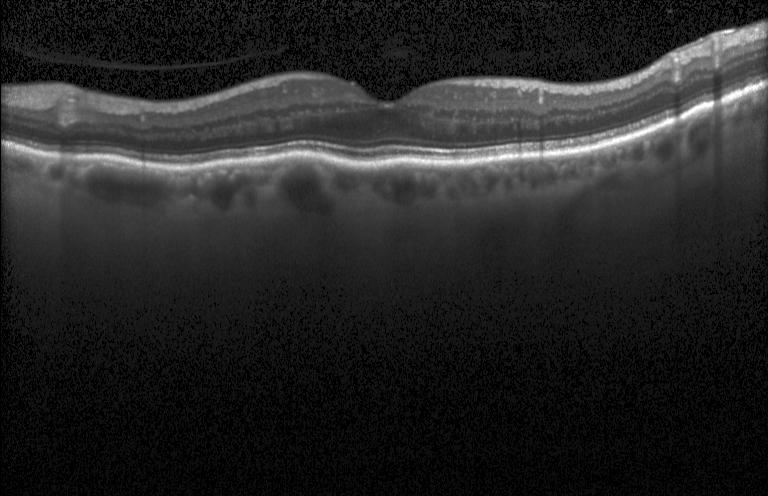 Retinal OCT cross-section showing neither choroidal neovascularization, diabetic macular edema, nor drusen.